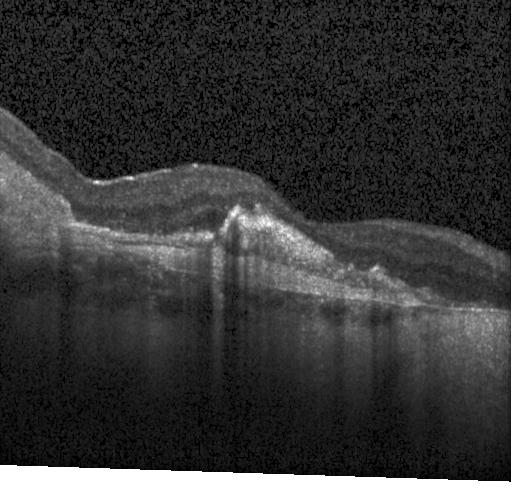
OCT scan showing choroidal neovascularization (CNV).